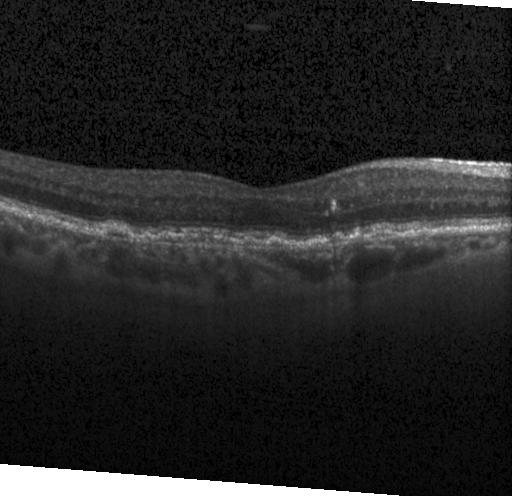

Spectral-domain optical coherence tomography, Heidelberg Spectralis, retinal OCT cross-section, centered on the fovea. Diagnosis: a choroidal neovascular membrane.